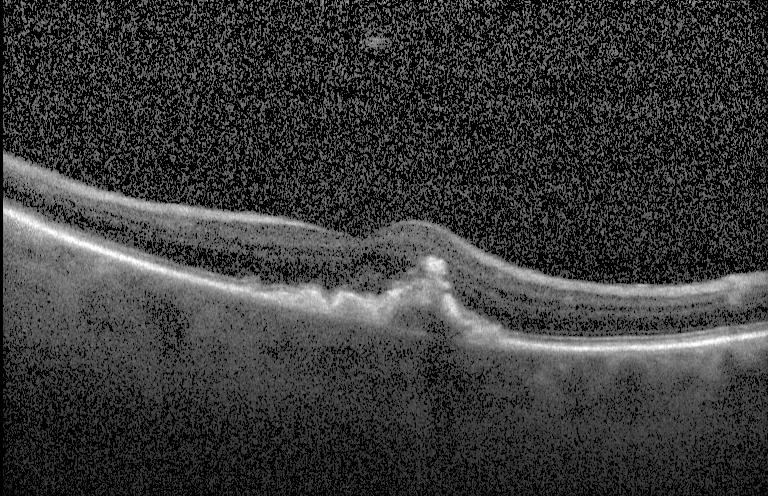

Optical coherence tomography scan · Heidelberg Spectralis. This B-scan demonstrates choroidal neovascularization (CNV).